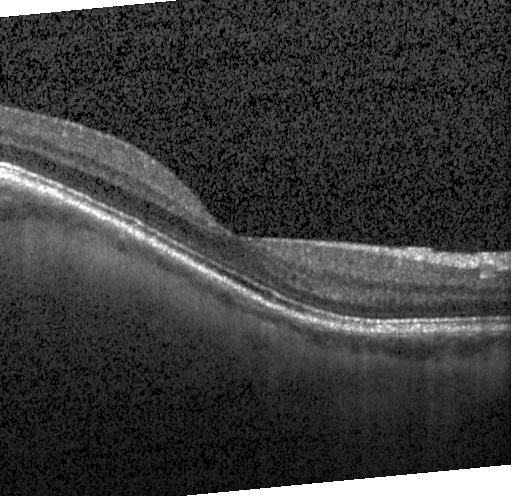
Macular OCT demonstrating neither CNV, DME, nor drusen.